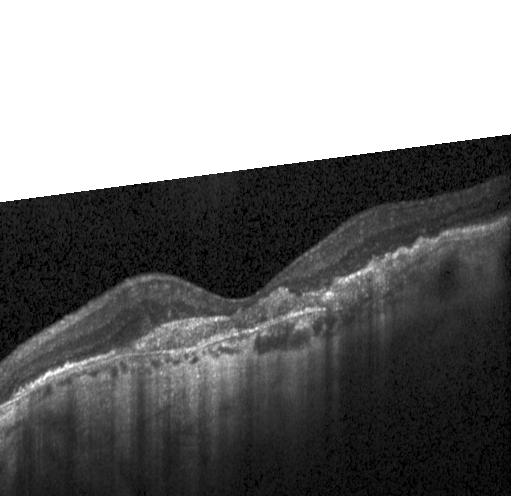 Macular OCT: choroidal neovascularization.